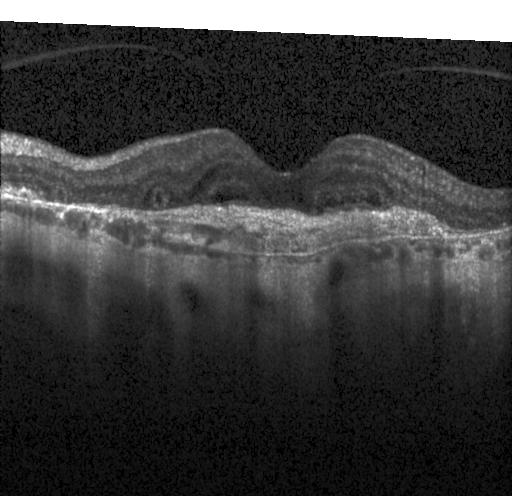 Optical coherence tomography scan
Assessment: choroidal neovascularization.